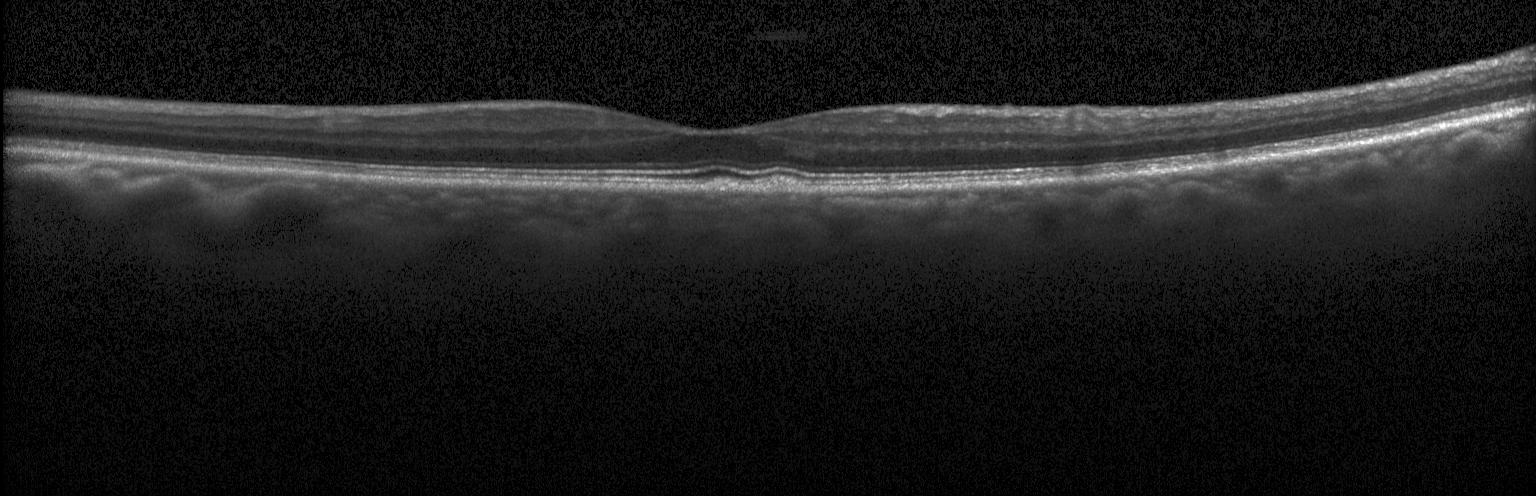
Instrument: Heidelberg Spectralis, spectral-domain OCT, OCT B-scan
Macular OCT: multiple drusen.